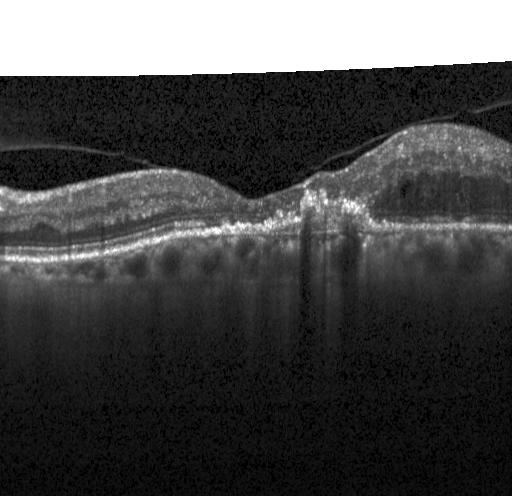 The scan shows choroidal neovascularization.